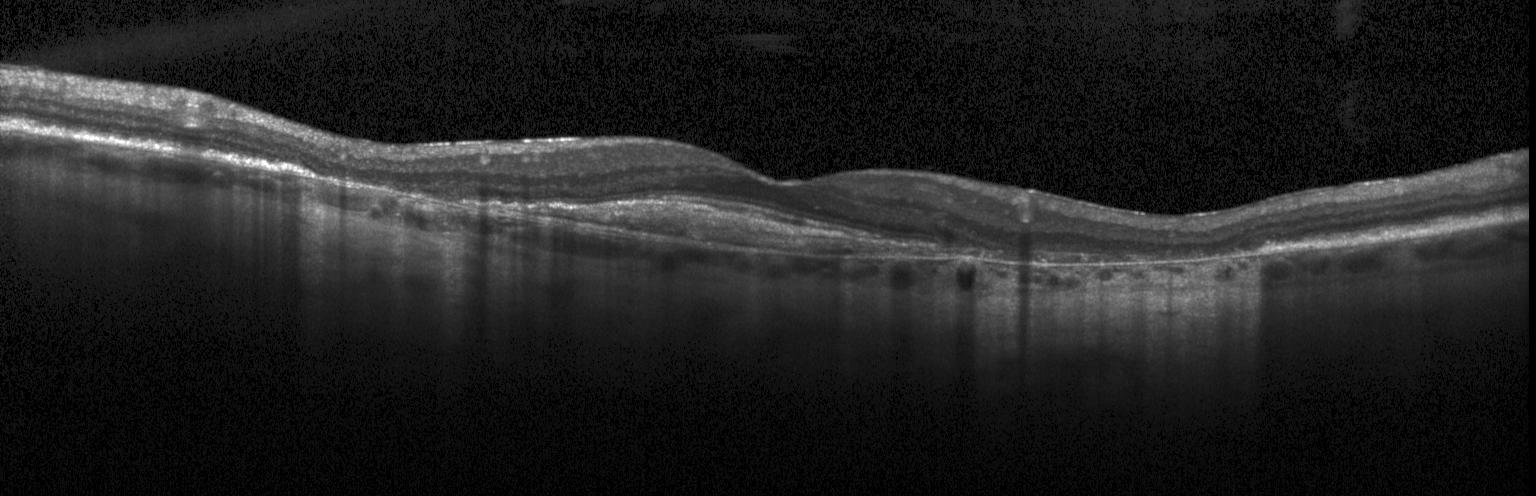

Macular OCT: CNV.